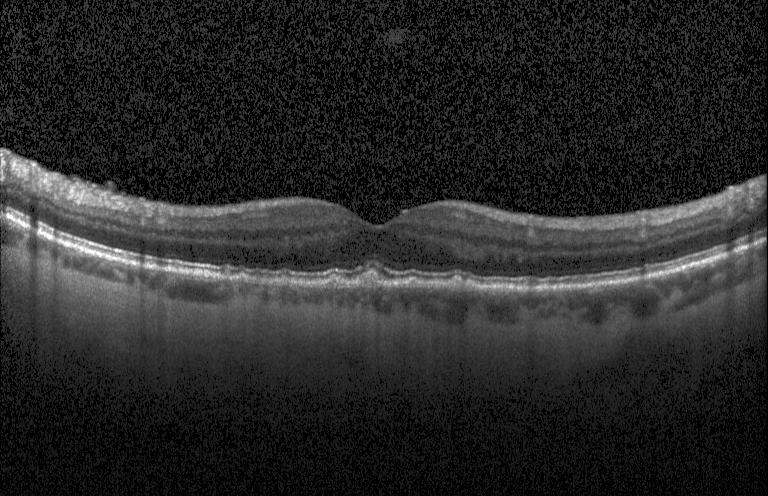 Impression: sub-RPE drusenoid deposits.